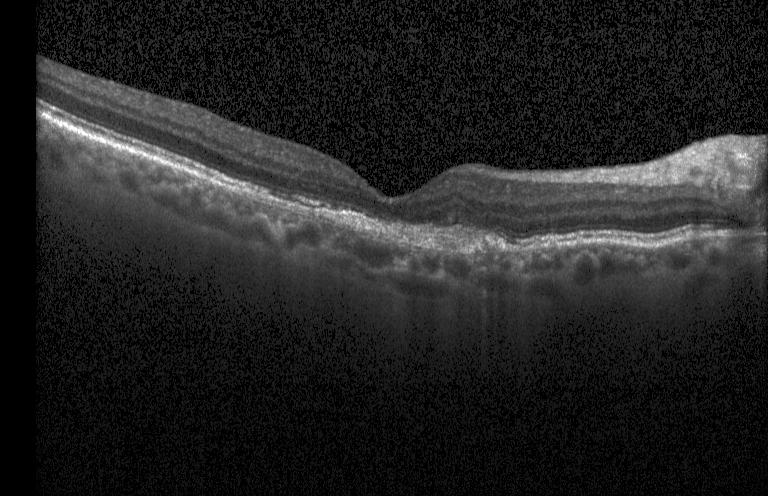 OCT finding: choroidal neovascularization.